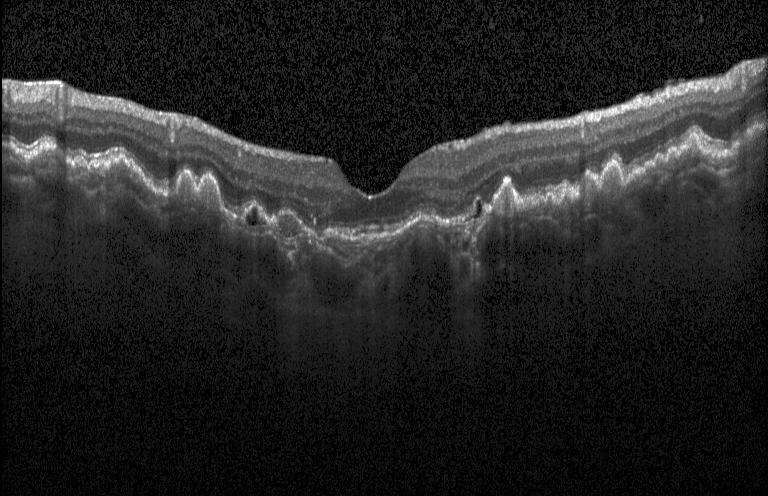

Retinal OCT cross-section · centered on the fovea · acquired on a Heidelberg Spectralis — Diagnosis: choroidal neovascularization.